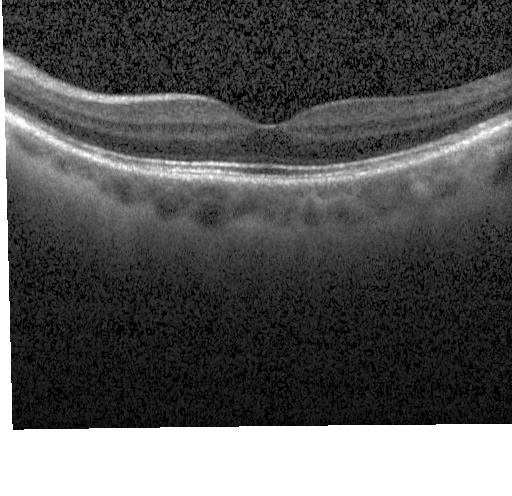

Retinal OCT cross-section · Heidelberg Spectralis. OCT finding: no choroidal neovascularization, diabetic macular edema, or drusen.